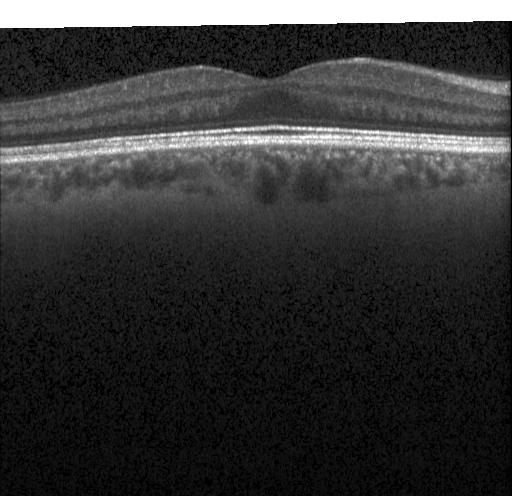
Optical coherence tomography B-scan — Macular OCT: no CNV, DME, or drusen.